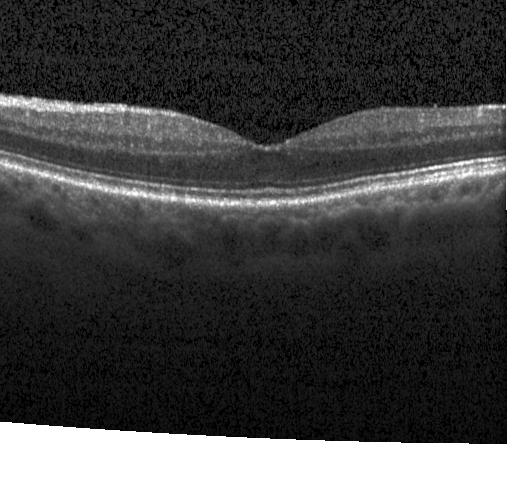

Optical coherence tomography scan. Impression: no choroidal neovascularization, no diabetic macular edema, and no drusen.